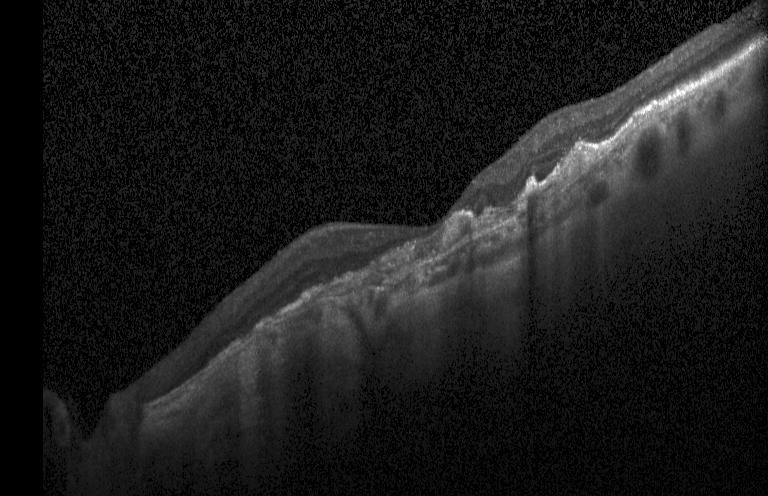 SD-OCT. Optical coherence tomography B-scan — This B-scan demonstrates choroidal neovascularization.